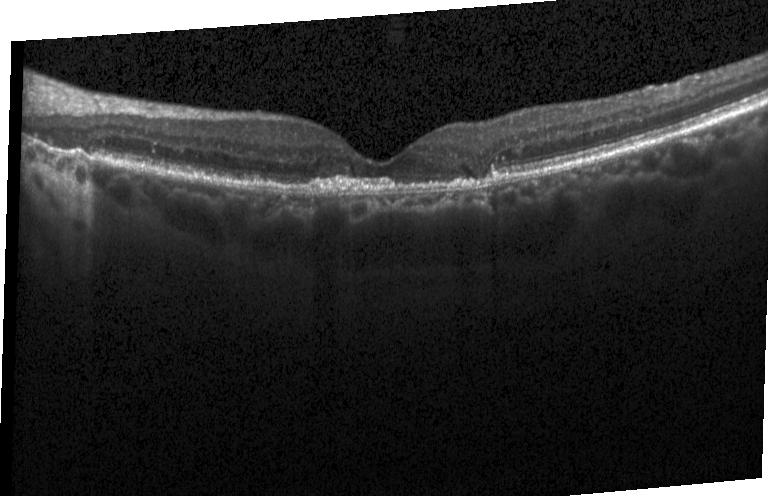

Spectral-domain OCT B-scan: CNV.